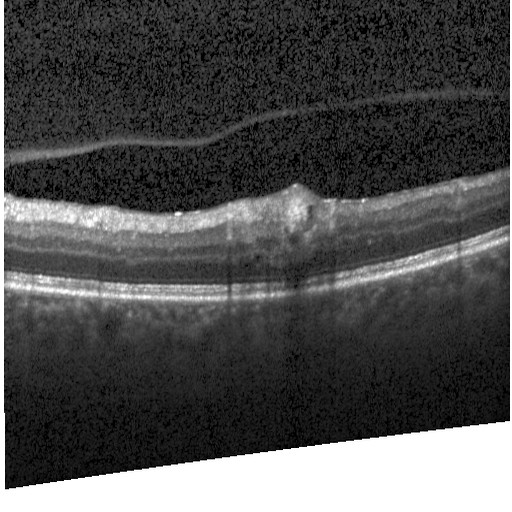 Centered on the fovea, retinal OCT B-scan — The scan shows diabetic macular edema.